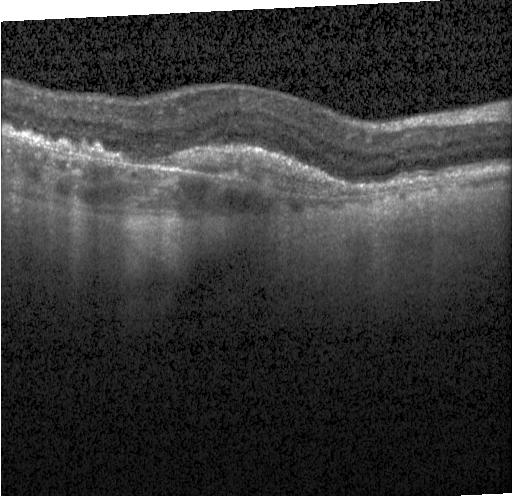 Horizontal scan through the fovea; spectral-domain optical coherence tomography; retinal OCT cross-section
Dx: a choroidal neovascular membrane.